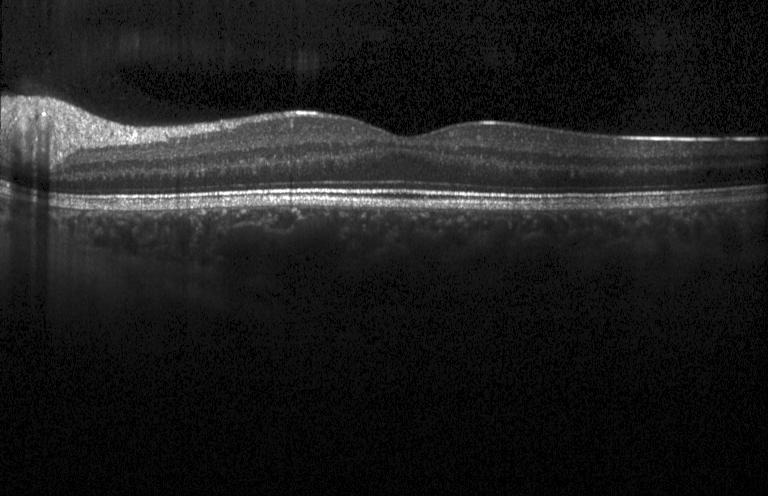 Macular OCT demonstrating no choroidal neovascularization, no diabetic macular edema, and no drusen.